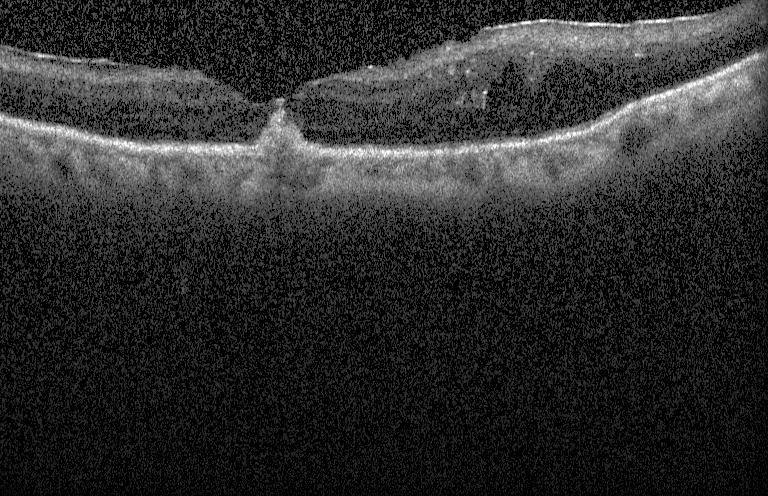 Diagnosis: CNV.